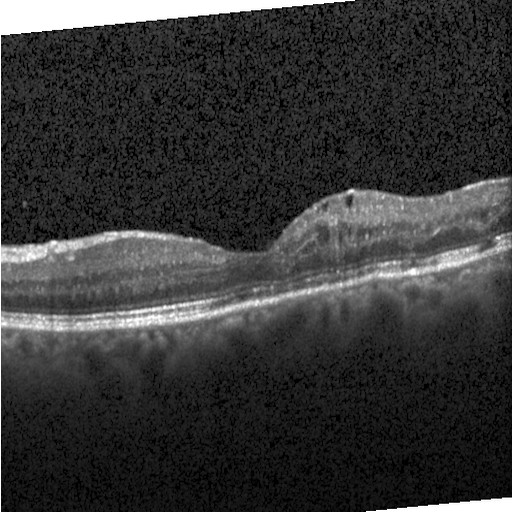 Impression: DME.